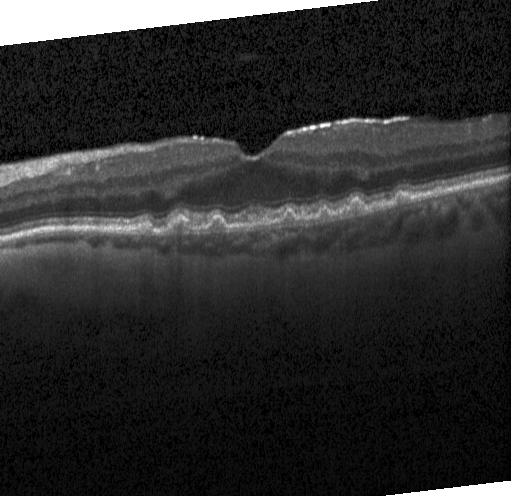
Optical coherence tomography B-scan, Heidelberg Spectralis OCT system, spectral-domain optical coherence tomography.
Macular OCT: multiple drusen.